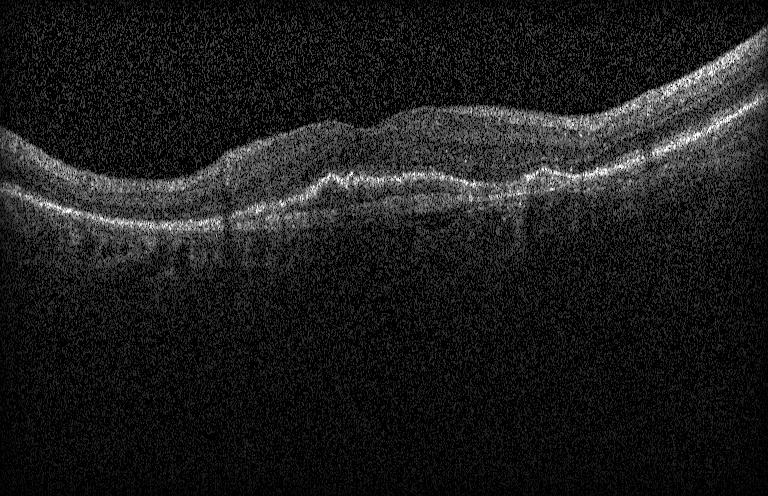

Dx: a choroidal neovascular membrane.